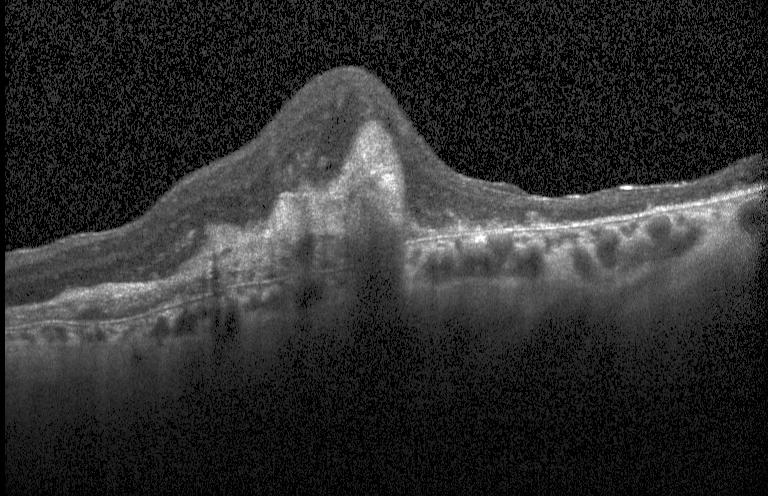

This B-scan demonstrates choroidal neovascularization (CNV).